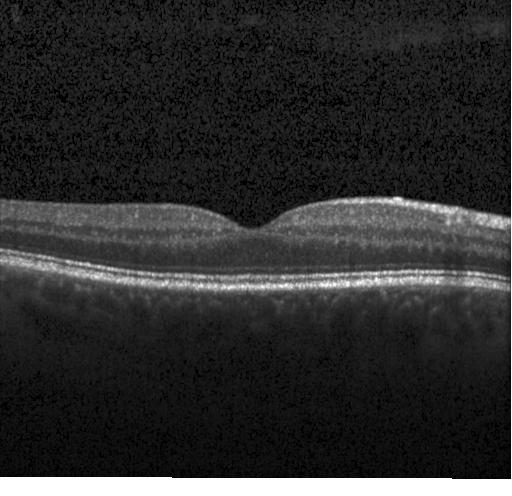
Instrument: Heidelberg Spectralis · spectral-domain OCT · OCT B-scan · centered on the fovea. OCT finding: neither choroidal neovascularization, diabetic macular edema, nor drusen.